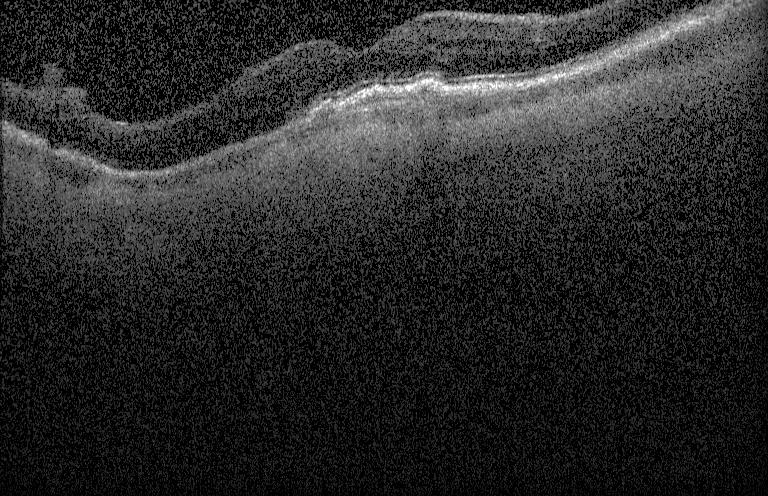

Spectral-domain OCT B-scan: a choroidal neovascular membrane.